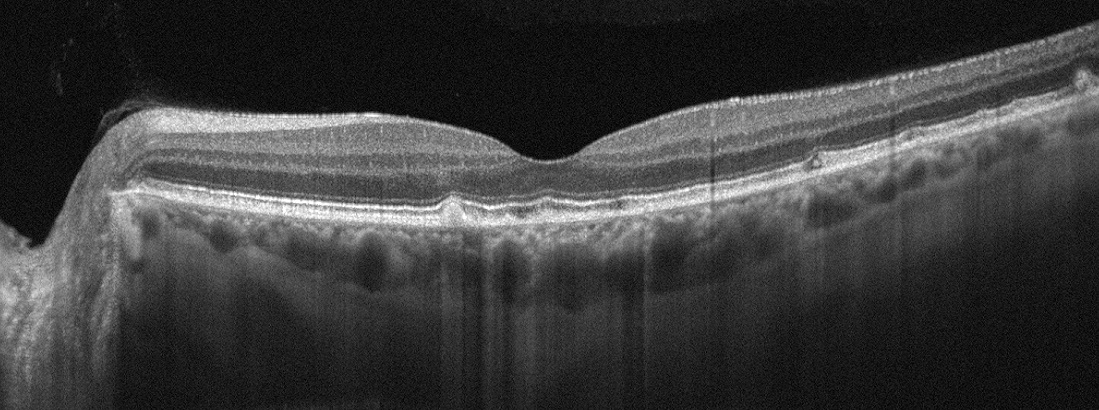 Acquired on an Optovue Avanti RTVue XR, retinal OCT cross-section, macular scan.
Finding: age-related macular degeneration.